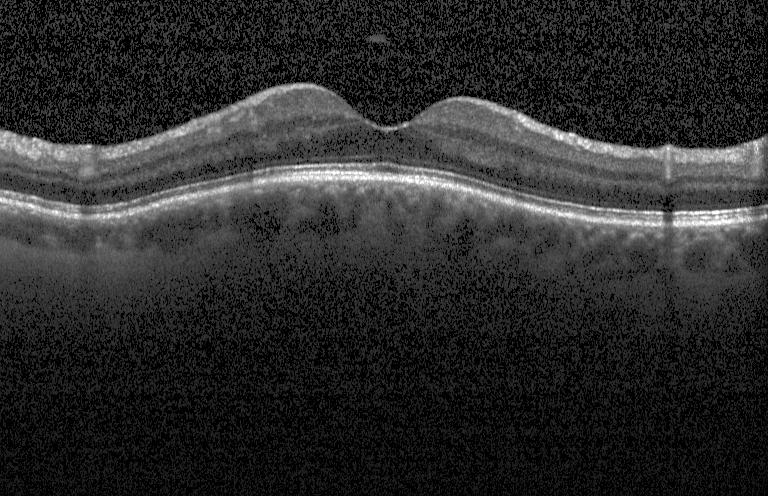 No choroidal neovascularization, no diabetic macular edema, and no drusen.